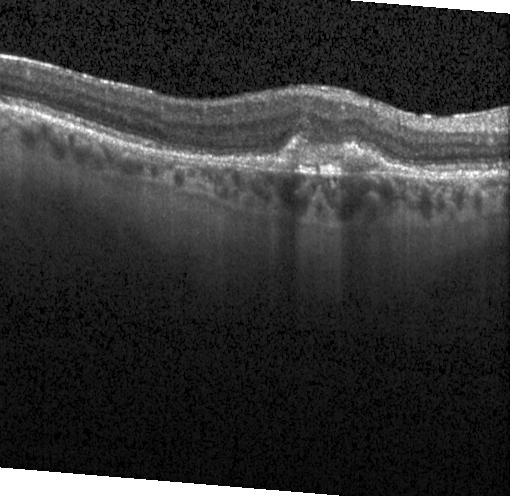

OCT B-scan · horizontal scan through the fovea · spectral-domain optical coherence tomography · Heidelberg Spectralis OCT system
Impression: choroidal neovascularization (CNV).